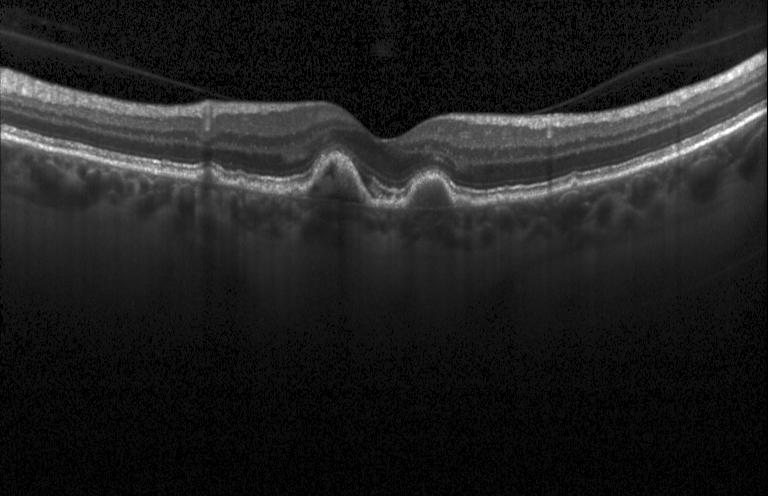

Spectral-domain OCT B-scan: drusen.